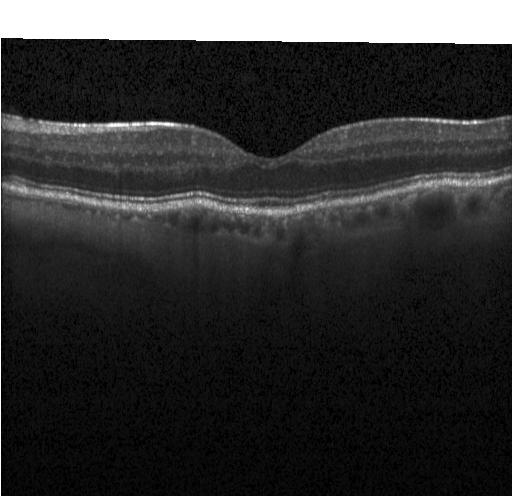
Macular scan · retinal OCT cross-section · spectral-domain OCT. This B-scan demonstrates no choroidal neovascularization, no diabetic macular edema, and no drusen.